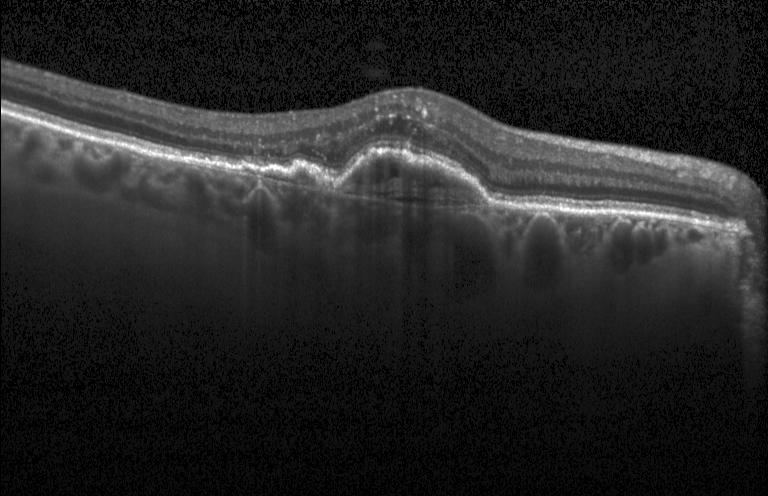 A choroidal neovascular membrane.